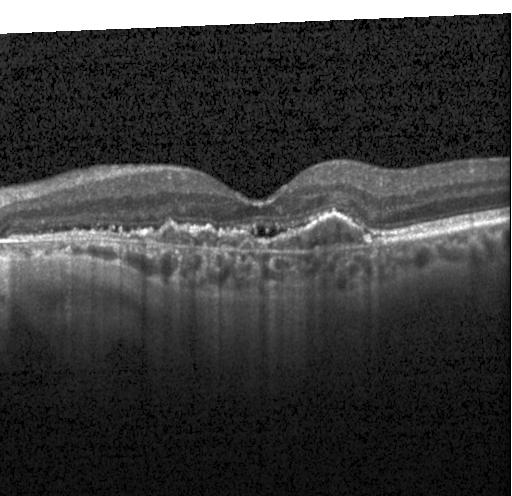

OCT scan showing a choroidal neovascular membrane.